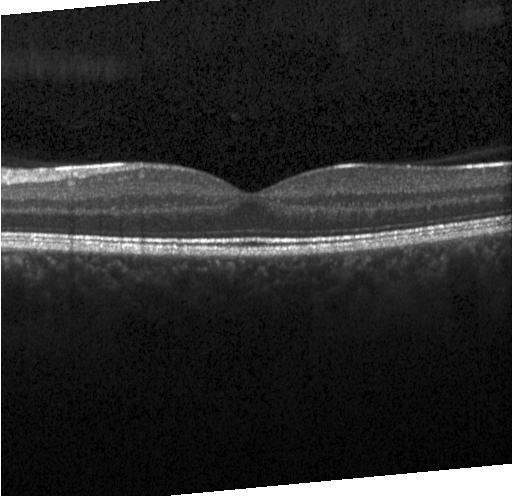

Assessment: no choroidal neovascularization, diabetic macular edema, or drusen.